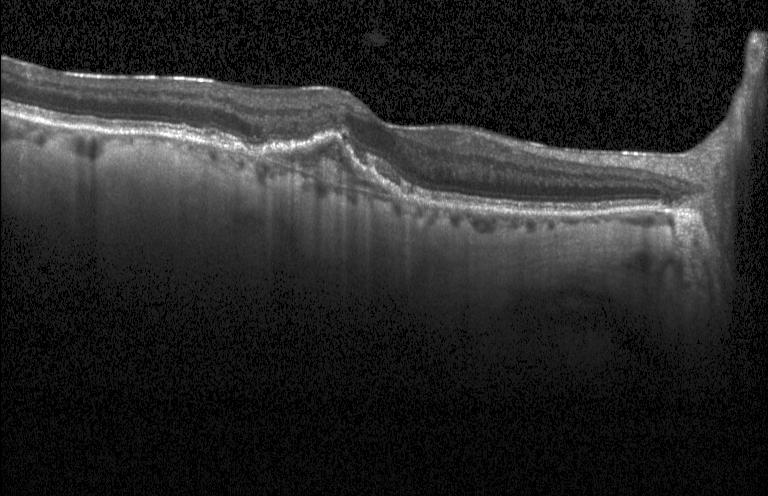 Spectral-domain OCT; retinal OCT B-scan — Dx: a choroidal neovascular membrane.